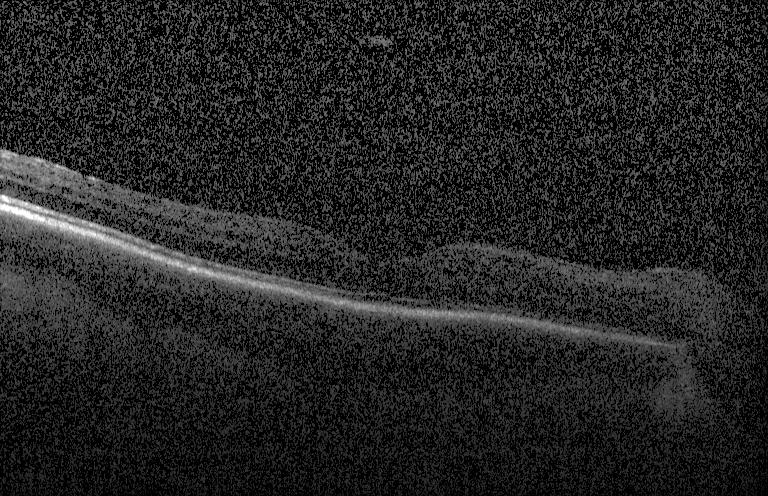

No CNV, DME, or drusen.